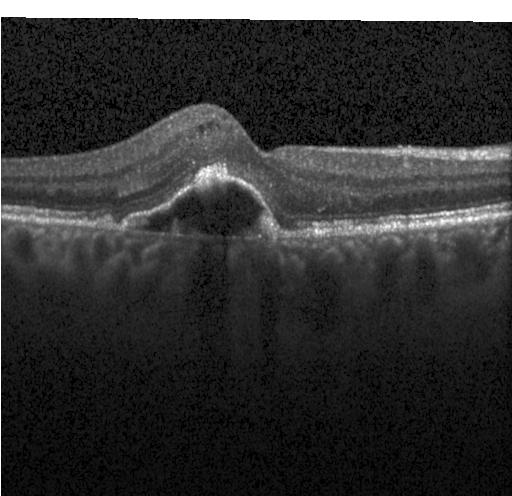 Finding: a choroidal neovascular membrane.